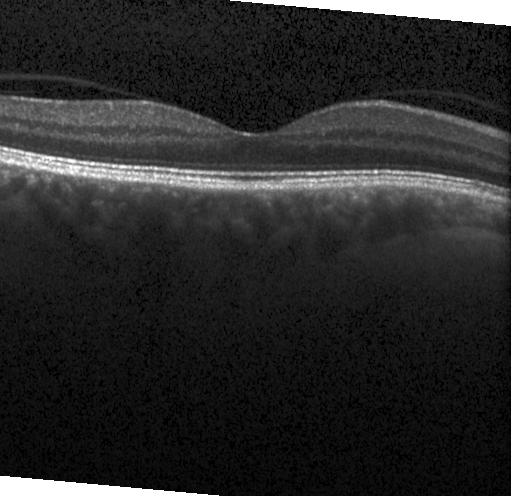

Spectral-domain optical coherence tomography · optical coherence tomography B-scan · Heidelberg Spectralis OCT system.
Dx: no choroidal neovascularization, diabetic macular edema, or drusen.